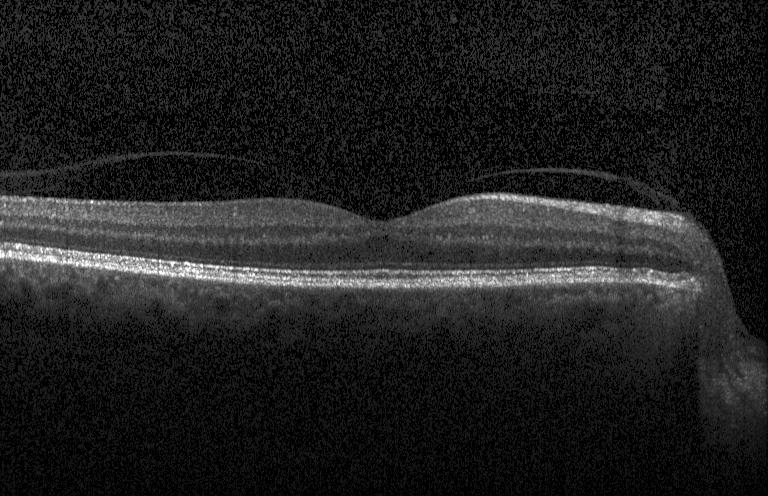
Impression: neither choroidal neovascularization, diabetic macular edema, nor drusen.